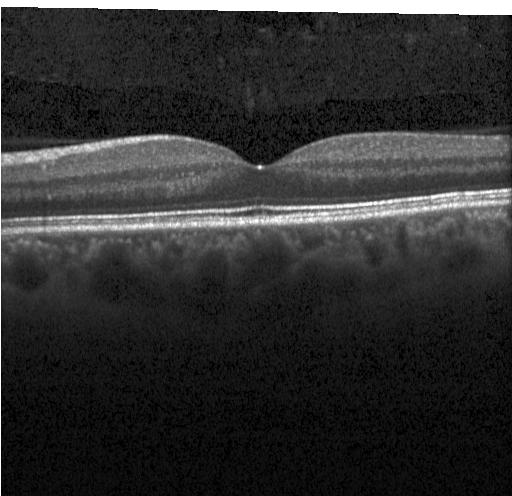
OCT B-scan showing no evidence of CNV, DME, or drusen.